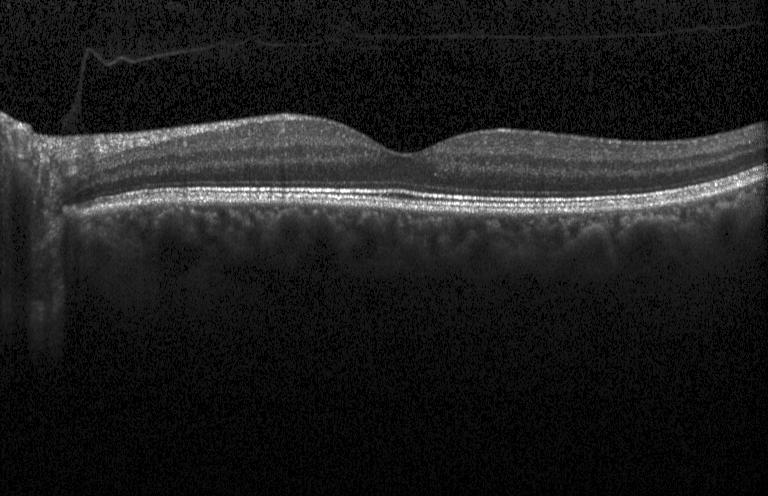

Optical coherence tomography B-scan
No choroidal neovascularization, diabetic macular edema, or drusen.